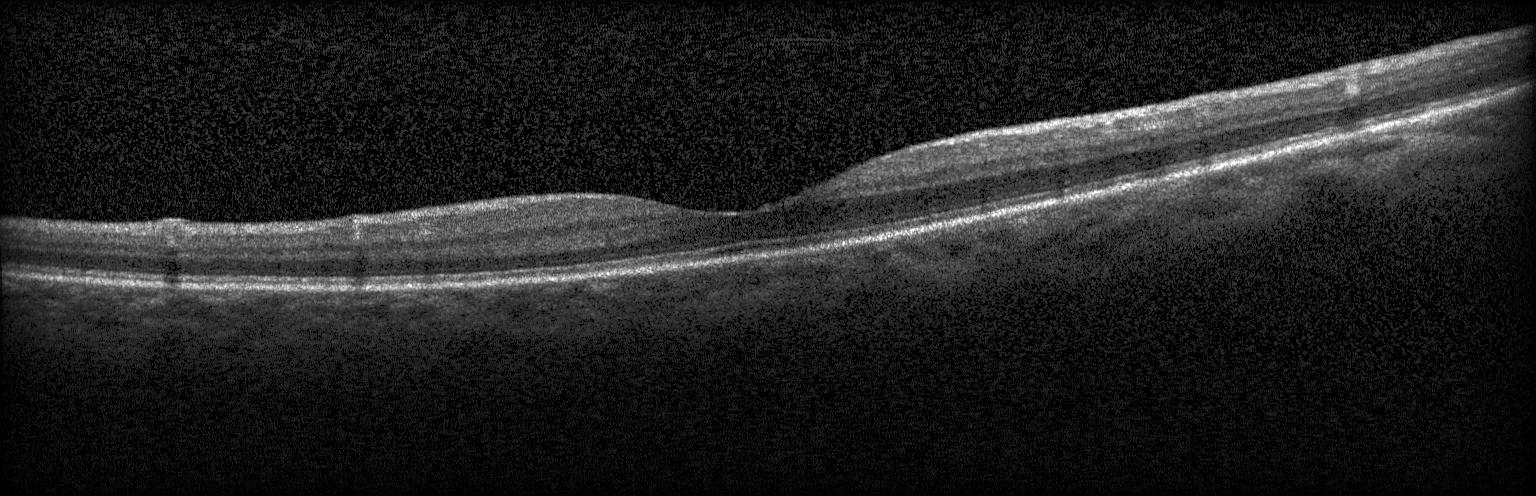 SD-OCT. Instrument: Heidelberg Spectralis. Centered on the fovea. OCT line scan. Assessment: no evidence of choroidal neovascularization, diabetic macular edema, or drusen.